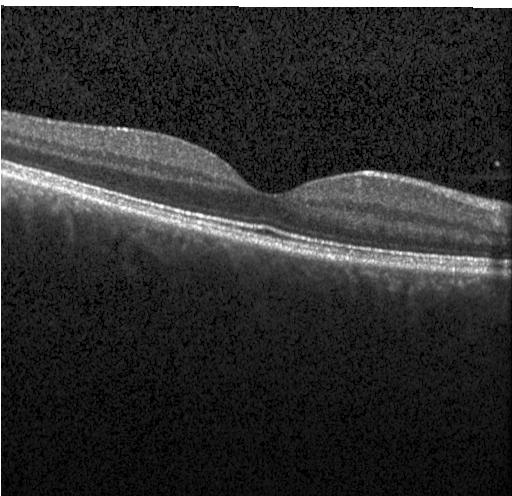
Heidelberg Spectralis OCT system · retinal OCT B-scan — Diagnosis: no choroidal neovascularization, diabetic macular edema, or drusen.